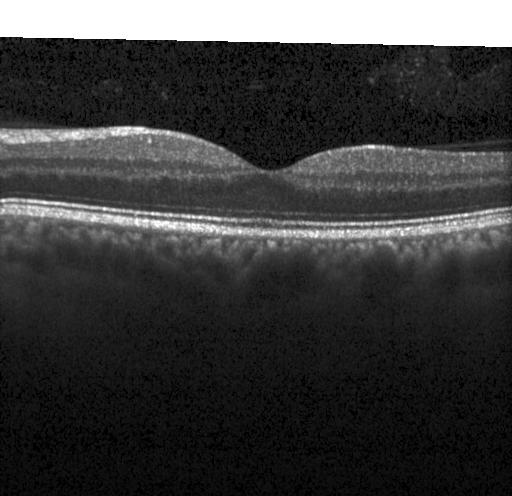
Instrument: Heidelberg Spectralis · retinal OCT B-scan.
Finding: no choroidal neovascularization, diabetic macular edema, or drusen.